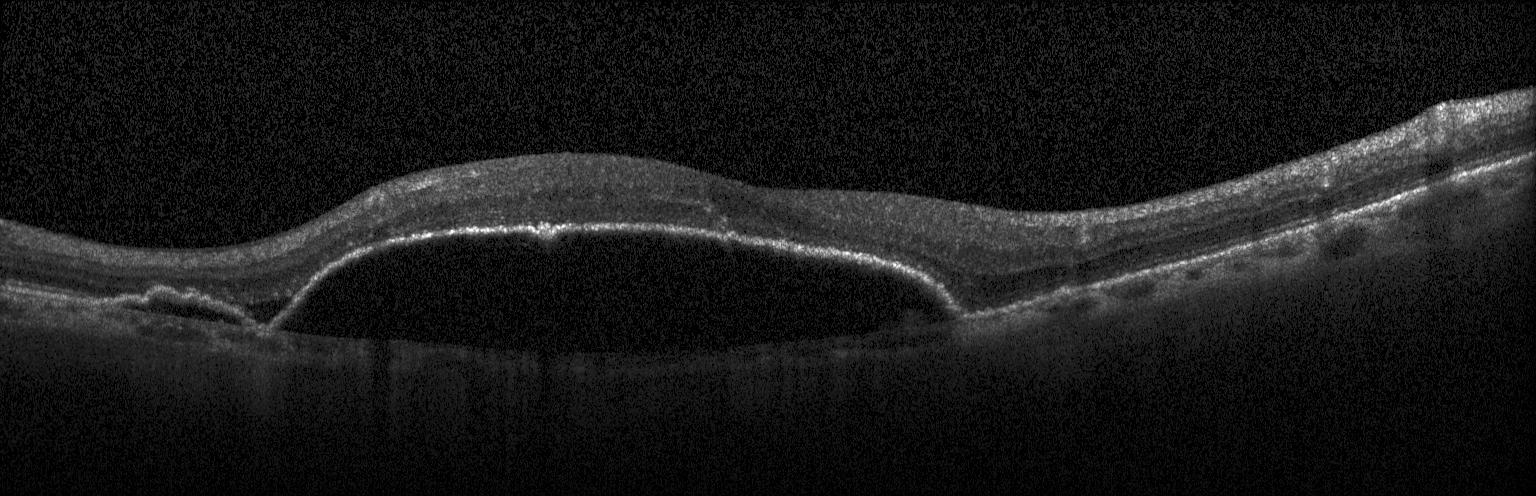 Dx: a choroidal neovascular membrane.